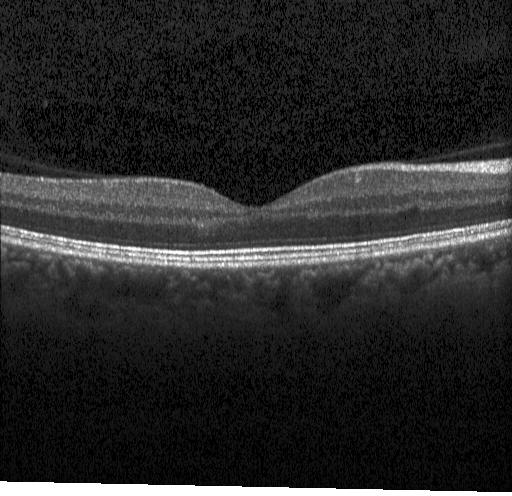
Spectral-domain optical coherence tomography; centered on the fovea; instrument: Heidelberg Spectralis; optical coherence tomography scan. Diagnosis: no evidence of choroidal neovascularization, diabetic macular edema, or drusen.